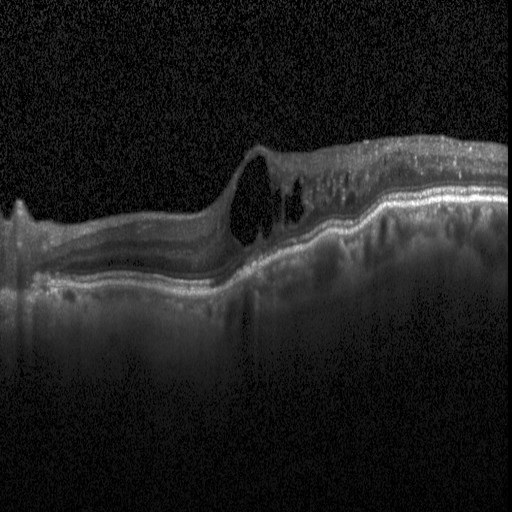
Spectral-domain OCT B-scan: DME.